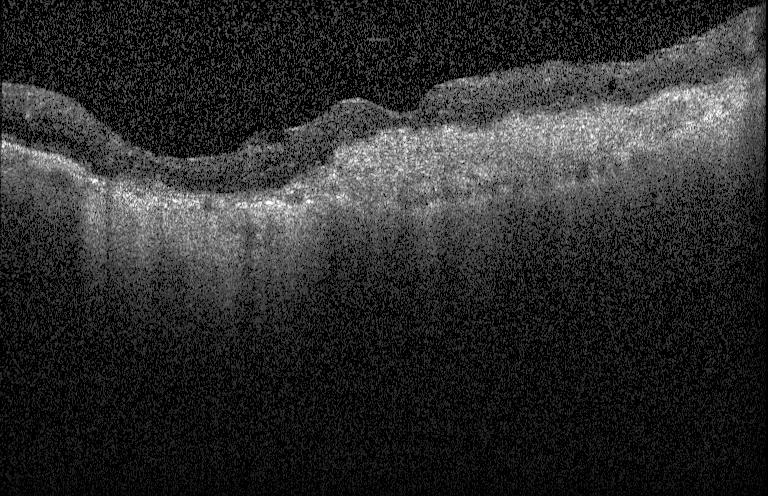
Optical coherence tomography B-scan
Diagnosis: choroidal neovascularization (CNV).